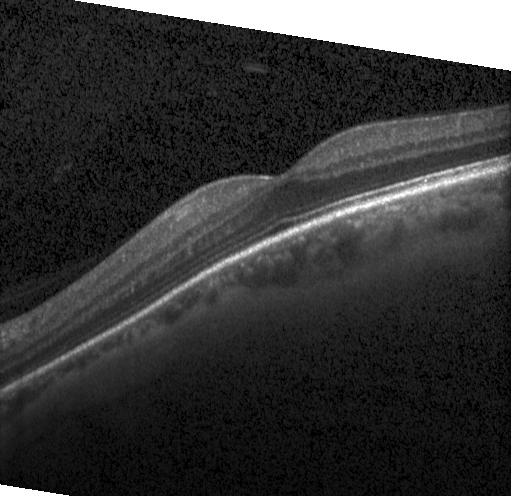

Optical coherence tomography B-scan. Horizontal scan through the fovea. Spectral-domain optical coherence tomography. Macular OCT: neither CNV, DME, nor drusen.